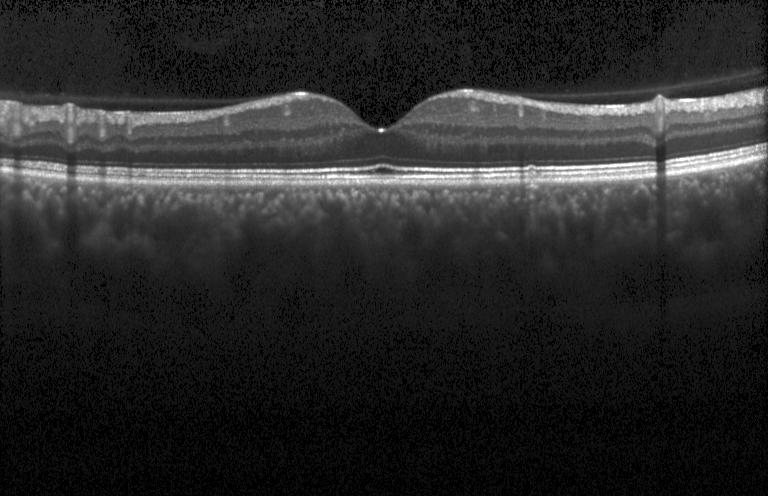

OCT line scan, macular scan
Dx: neither choroidal neovascularization, diabetic macular edema, nor drusen.